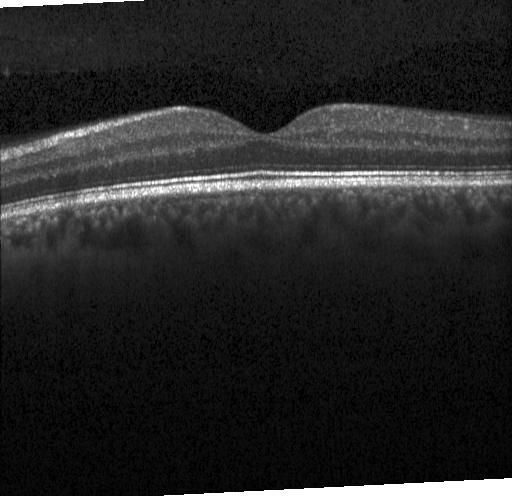 OCT line scan — Assessment: no evidence of choroidal neovascularization, diabetic macular edema, or drusen.